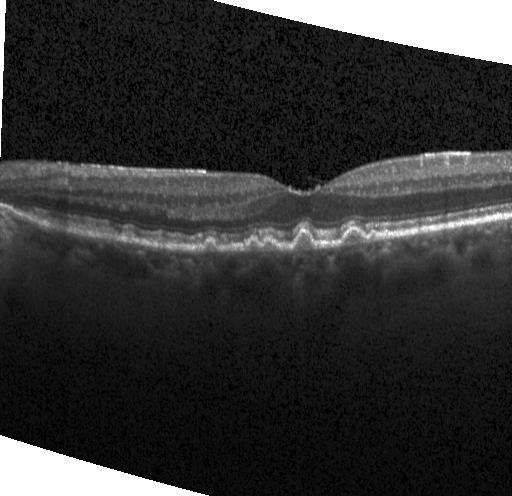 Macular OCT demonstrating sub-RPE drusenoid deposits.